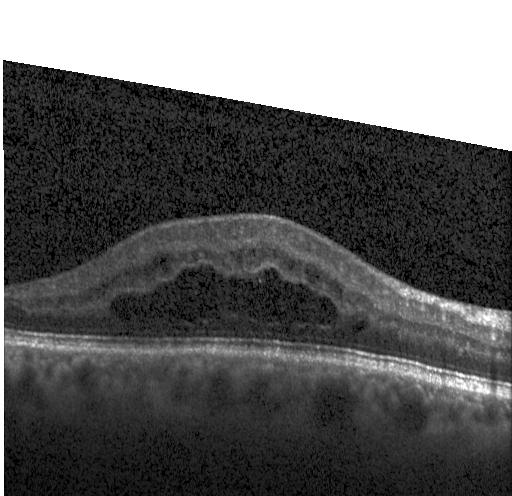
Heidelberg Spectralis, retinal OCT cross-section — The scan shows diabetic macular edema.